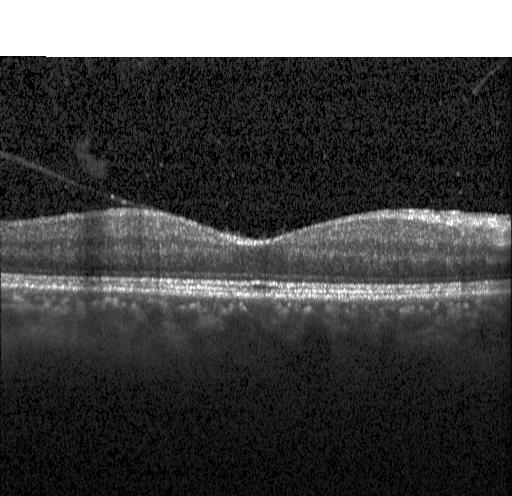
Optical coherence tomography scan, spectral-domain OCT
No choroidal neovascularization, no diabetic macular edema, and no drusen.